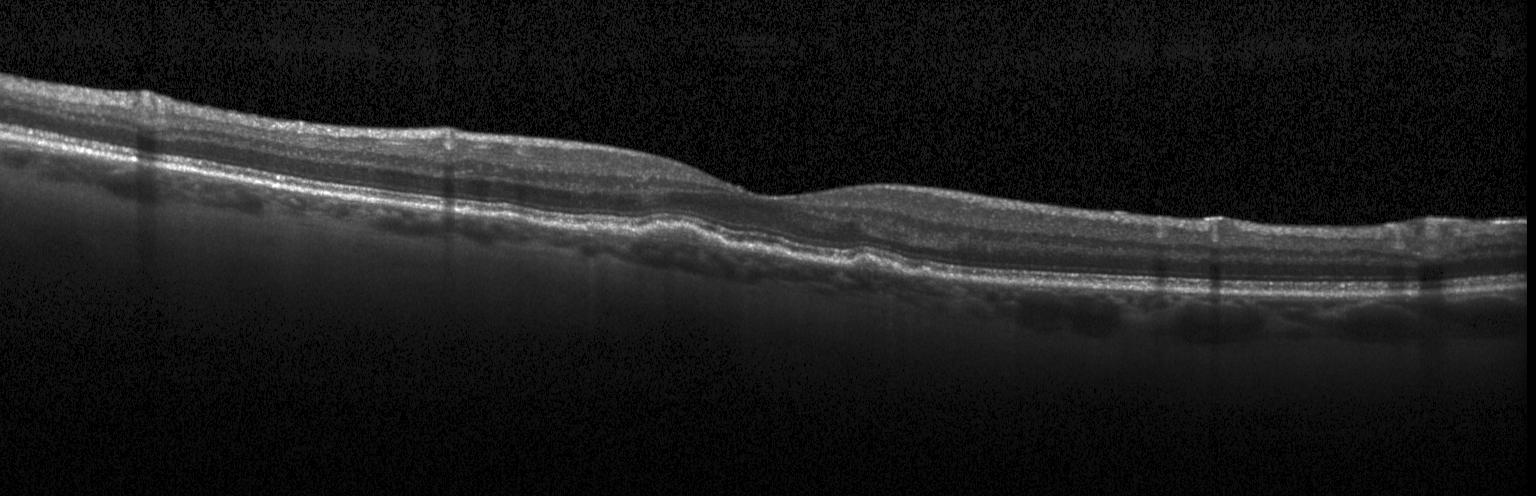
Optical coherence tomography scan · SD-OCT · centered on the fovea · Heidelberg Spectralis
Diagnosis: drusen.